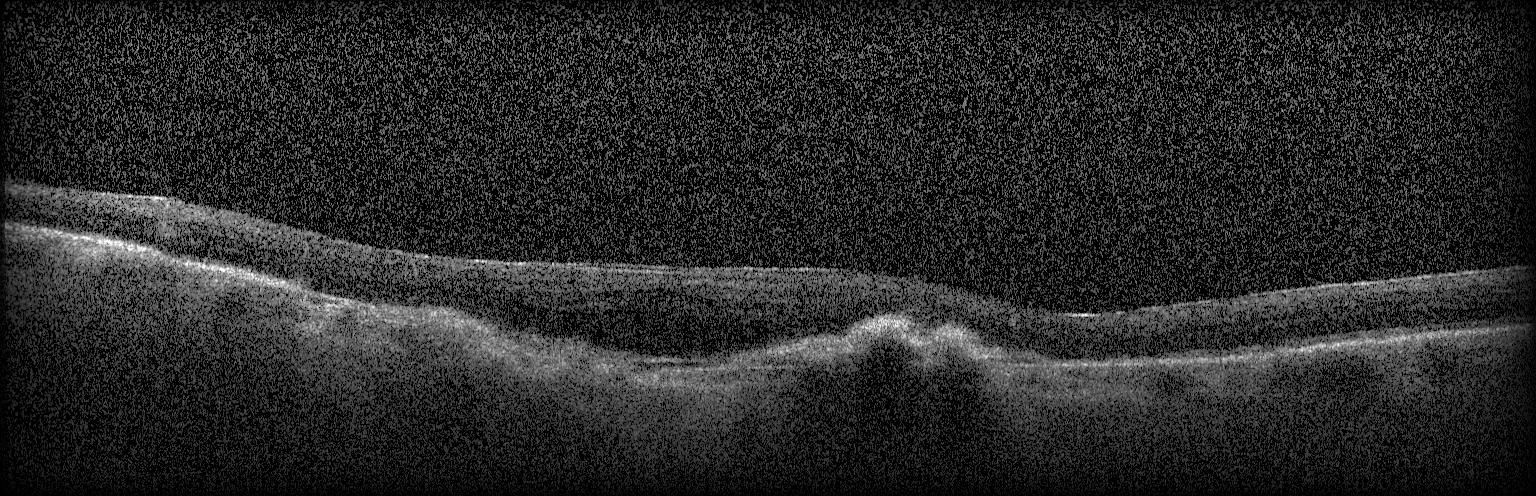
OCT B-scan; Heidelberg Spectralis
Choroidal neovascularization (CNV).